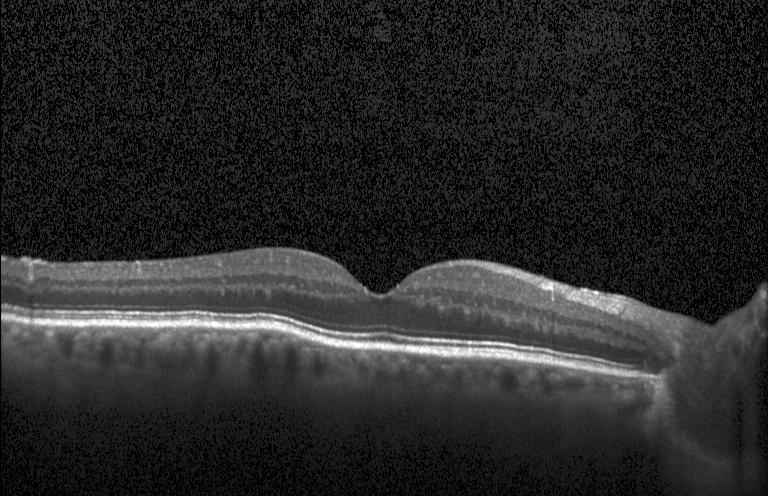
Optical coherence tomography B-scan
Dx: no CNV, DME, or drusen.